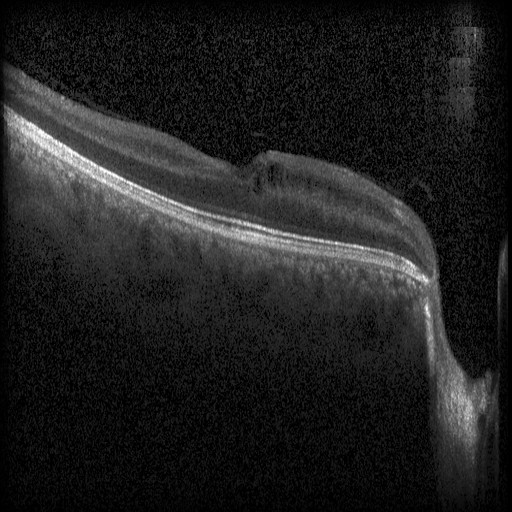 Diagnosis: diabetic macular edema (DME).